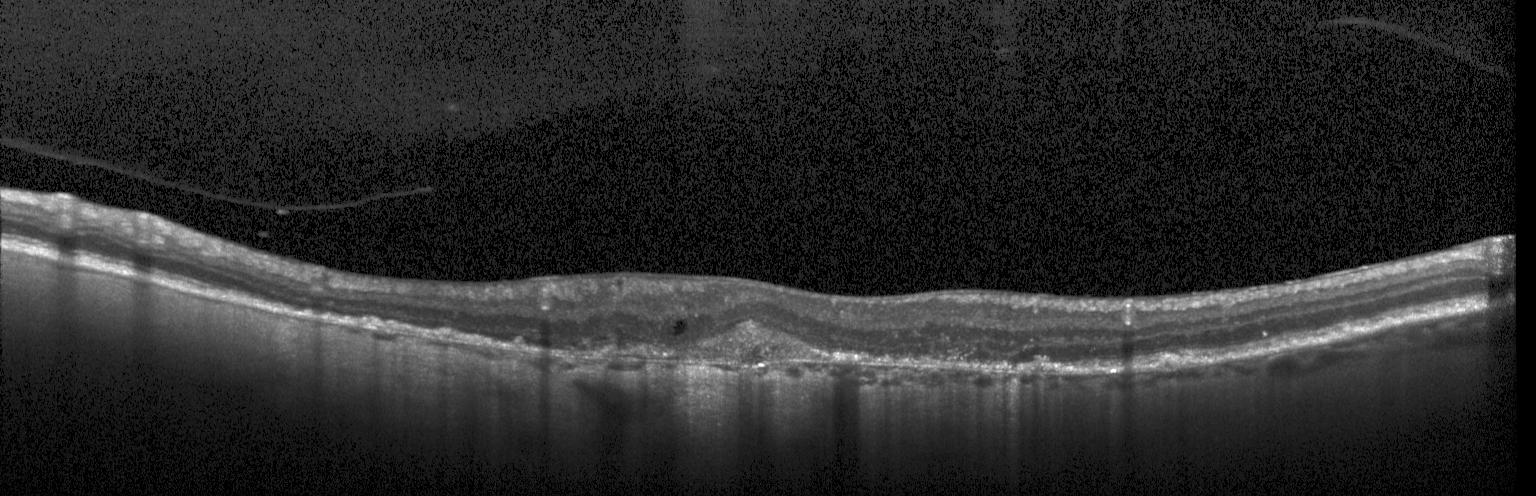 Retinal OCT B-scan, acquired on a Heidelberg Spectralis, macular scan.
Finding: choroidal neovascularization (CNV).